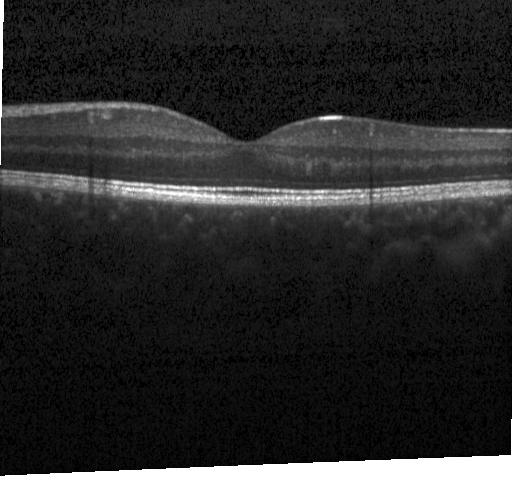

Optical coherence tomography scan
Impression: no CNV, DME, or drusen.